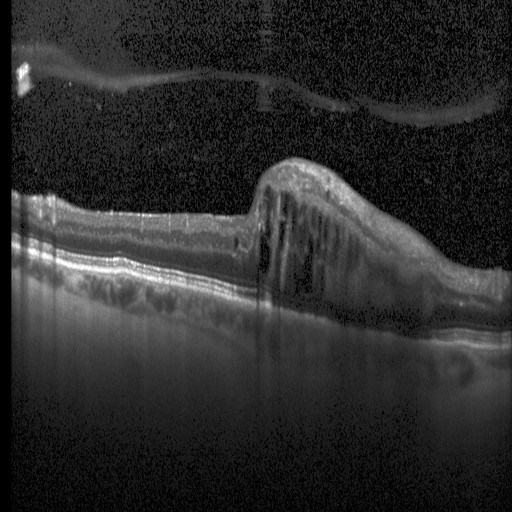

Finding: diabetic macular edema.